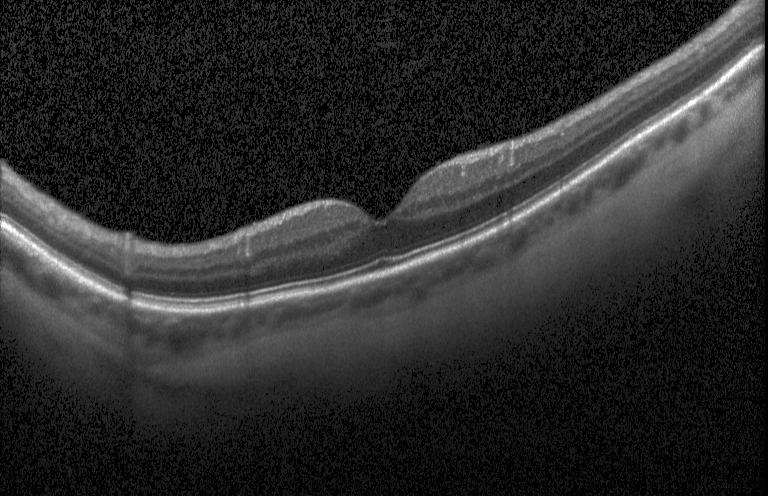

Assessment: no CNV, no DME, and no drusen.